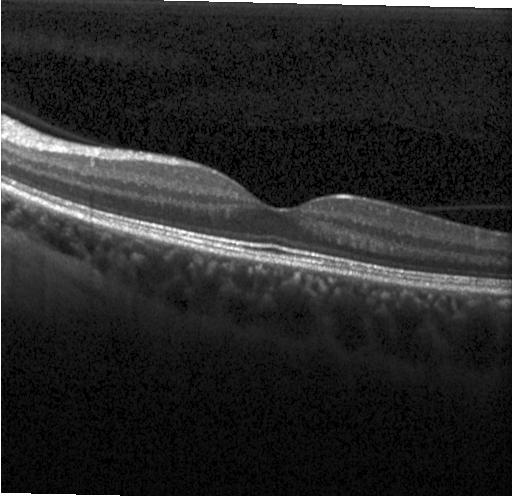

Diagnosis: no choroidal neovascularization, no diabetic macular edema, and no drusen.